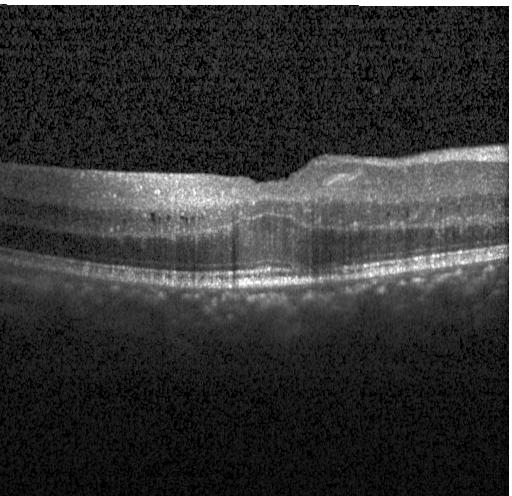
Optical coherence tomography scan. Centered on the fovea — Diabetic macular edema (DME).